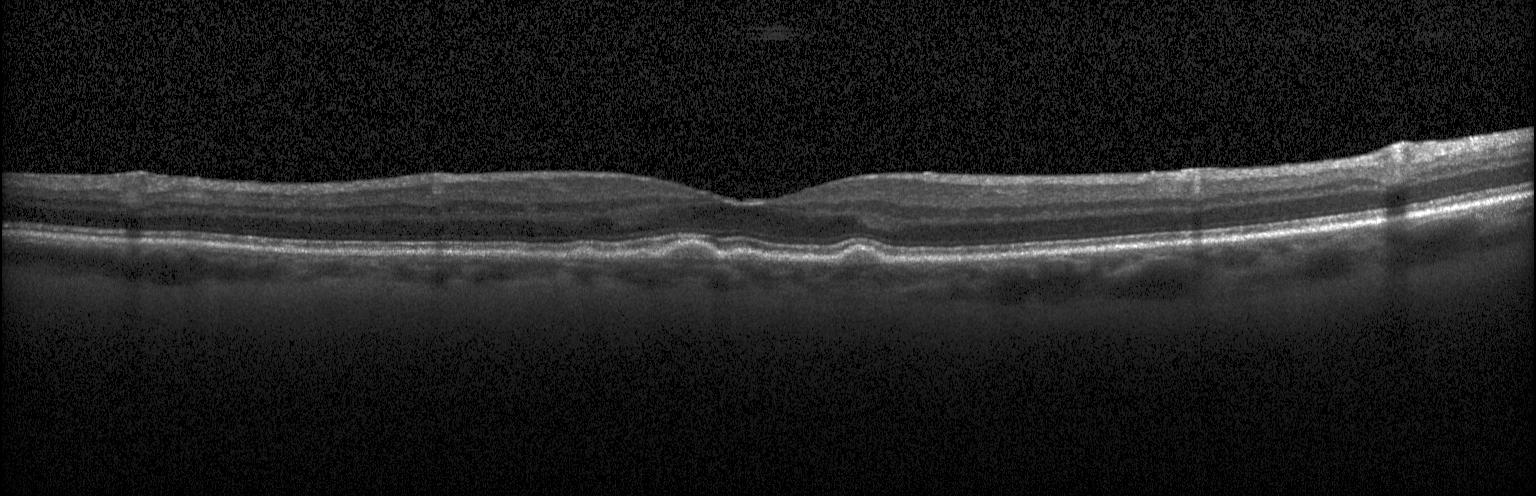 Optical coherence tomography B-scan, spectral-domain optical coherence tomography, Heidelberg Spectralis OCT system, through the macula
OCT finding: sub-RPE drusenoid deposits.